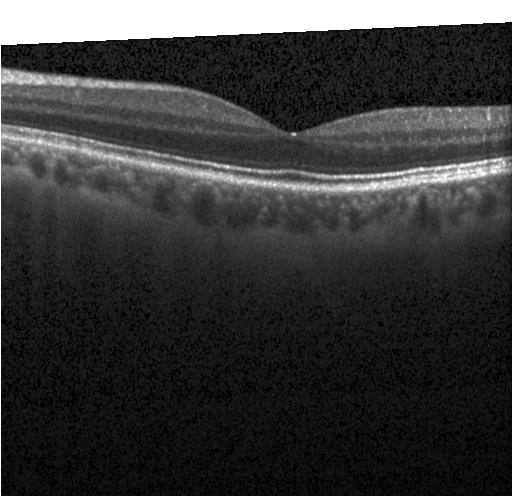
Through the macula. Heidelberg Spectralis OCT system. Optical coherence tomography scan. SD-OCT. The scan shows neither choroidal neovascularization, diabetic macular edema, nor drusen.